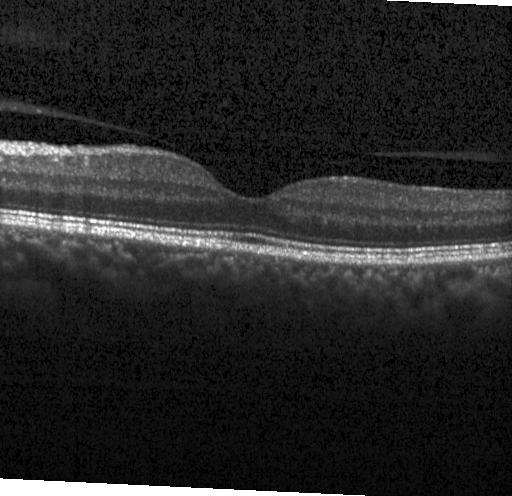 Heidelberg Spectralis OCT system. Spectral-domain OCT. Retinal OCT cross-section. Centered on the fovea. Finding: neither choroidal neovascularization, diabetic macular edema, nor drusen.